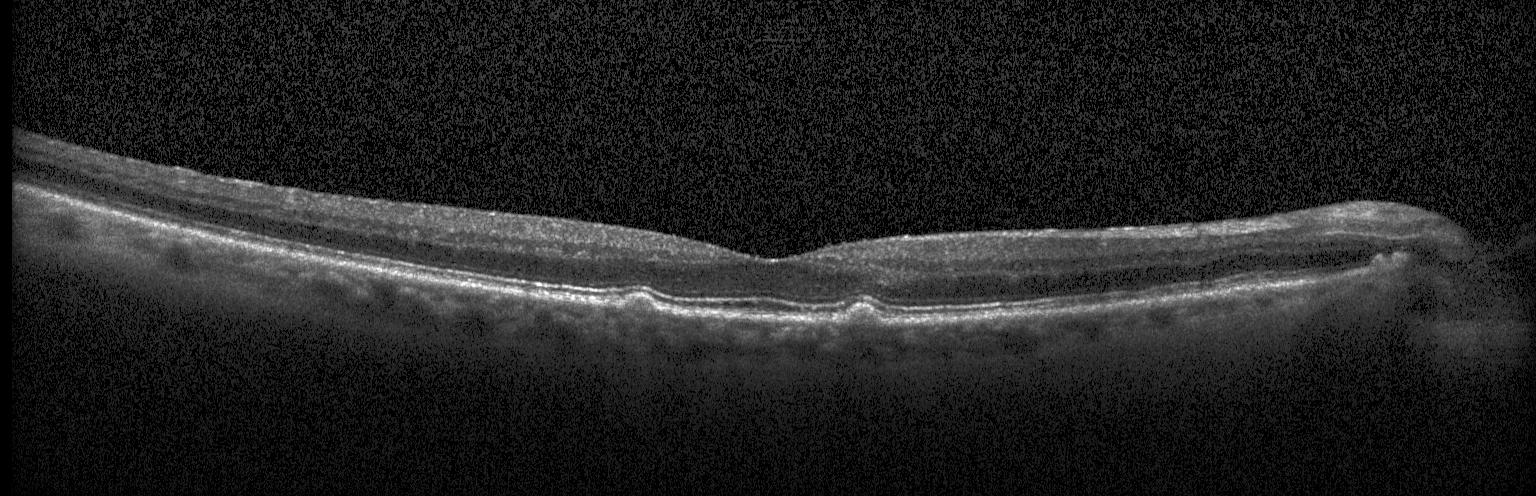 Optical coherence tomography B-scan
Finding: sub-RPE drusenoid deposits.